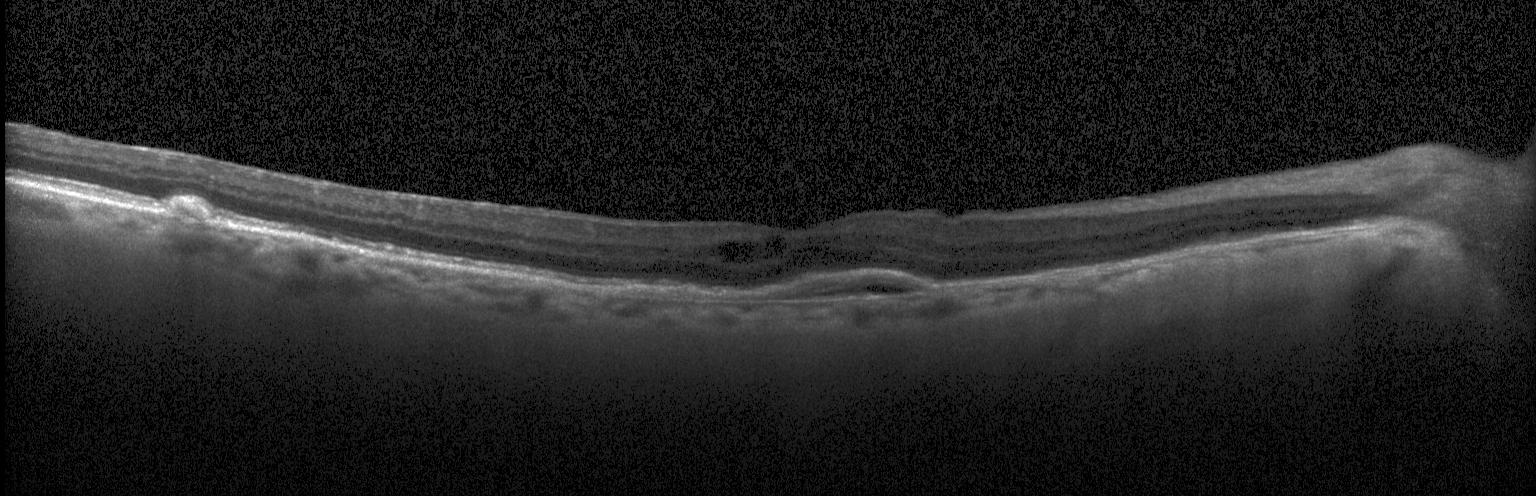

Choroidal neovascularization.